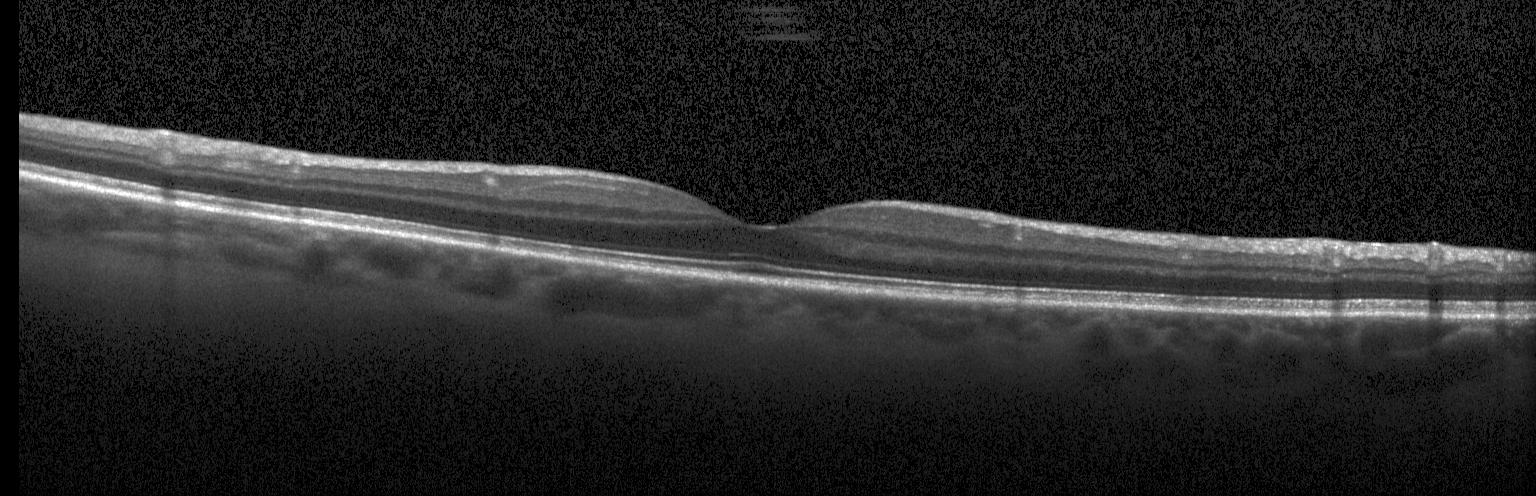 SD-OCT; acquired on a Heidelberg Spectralis; OCT B-scan
Diagnosis: no choroidal neovascularization, diabetic macular edema, or drusen.